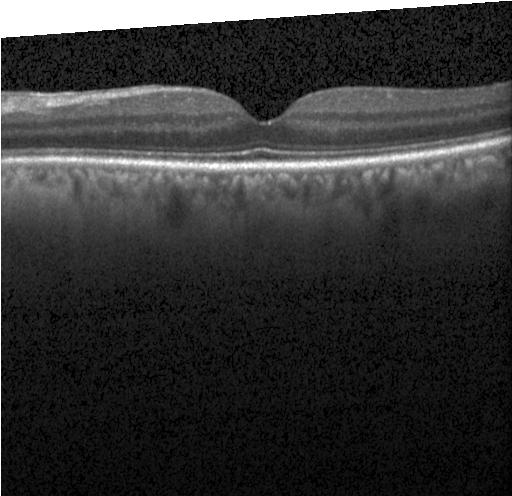

Retinal OCT cross-section showing no choroidal neovascularization, no diabetic macular edema, and no drusen.